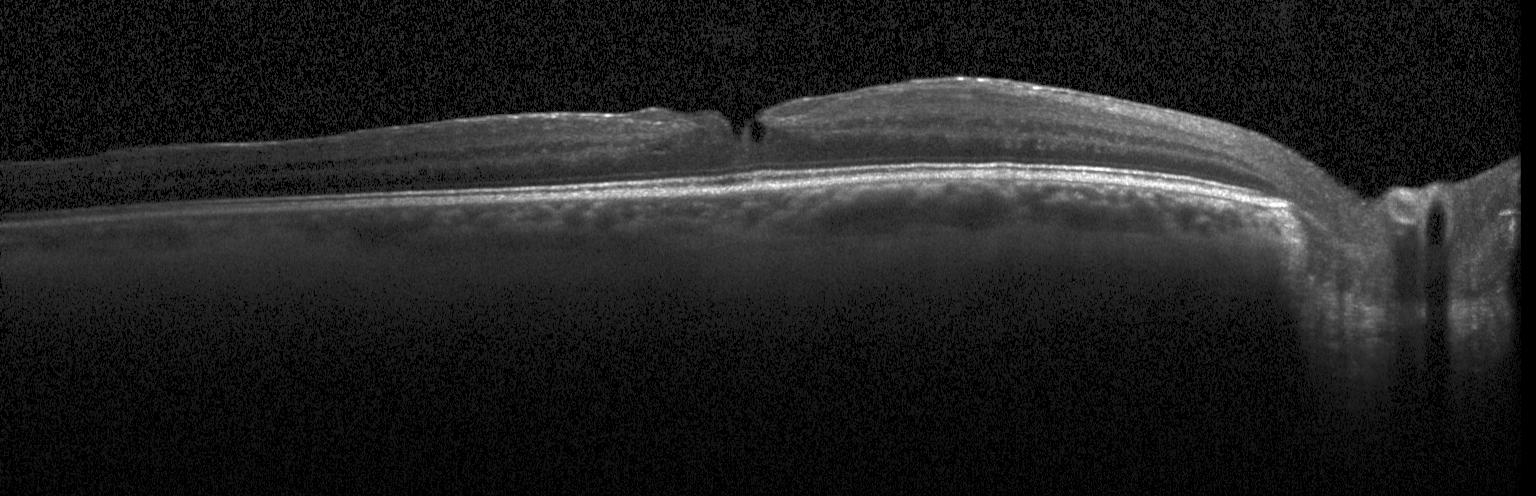 Optical coherence tomography scan, Heidelberg Spectralis. Diabetic macular edema (DME).